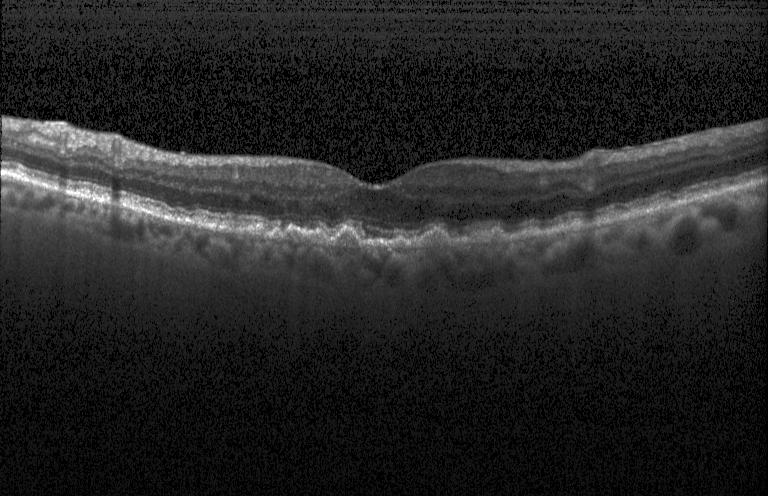 Retinal OCT B-scan. Fovea-centered. Instrument: Heidelberg Spectralis.
This B-scan demonstrates sub-RPE drusenoid deposits.